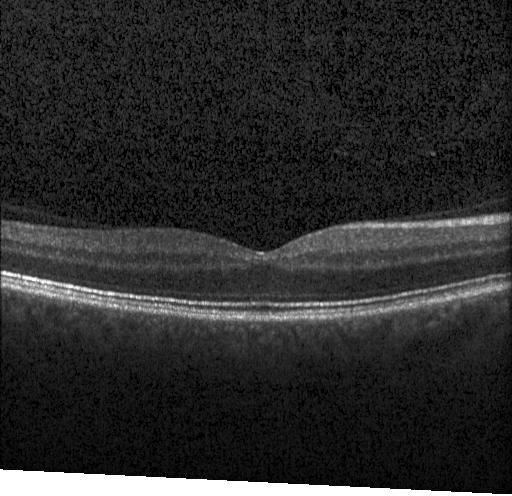

Spectral-domain OCT B-scan: no choroidal neovascularization, no diabetic macular edema, and no drusen.